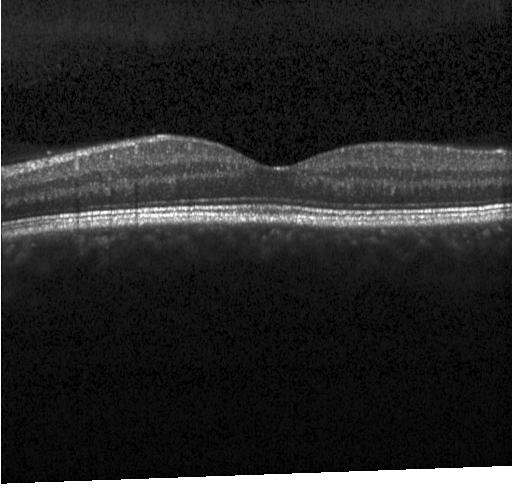

No choroidal neovascularization, diabetic macular edema, or drusen.